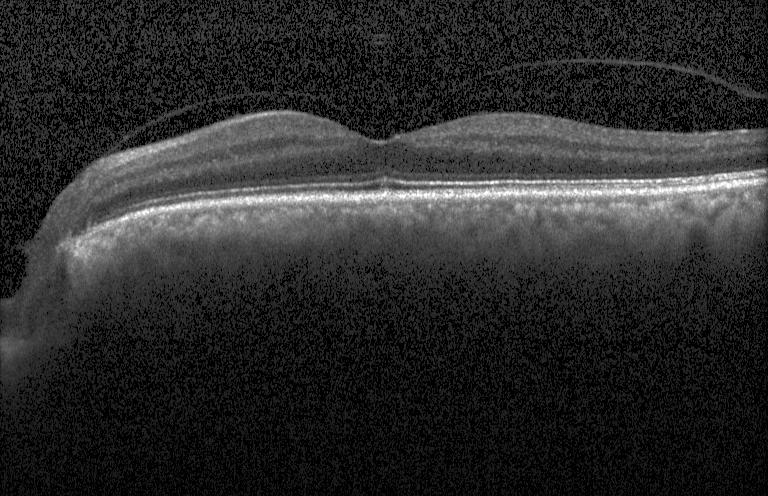 Finding: no choroidal neovascularization, diabetic macular edema, or drusen.